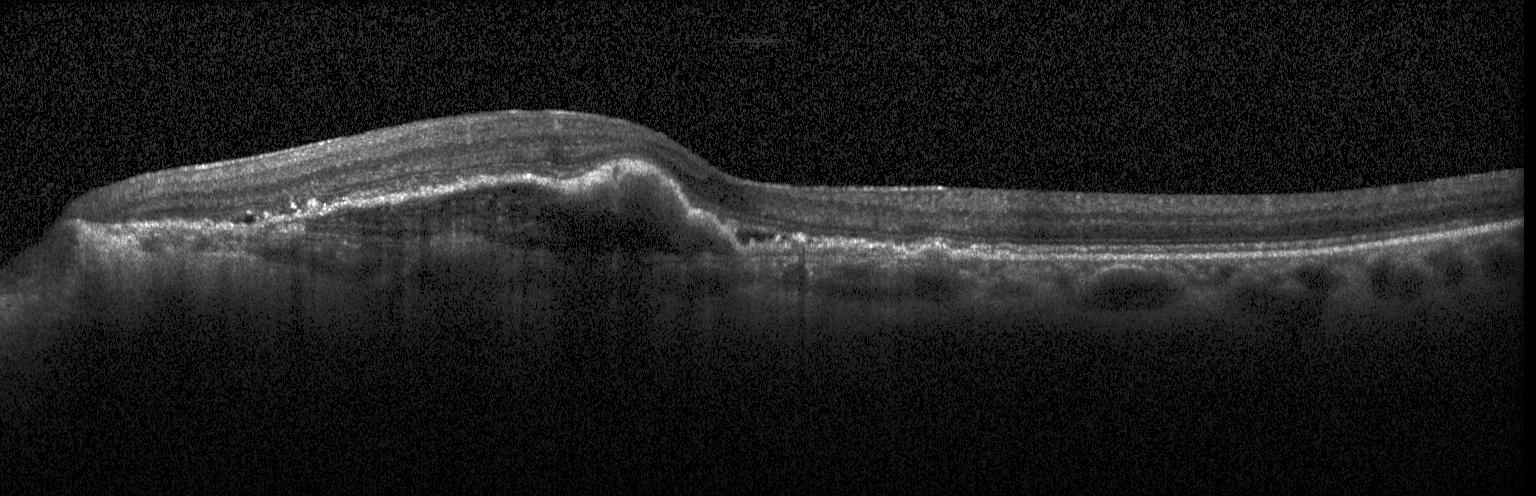
OCT finding: CNV.